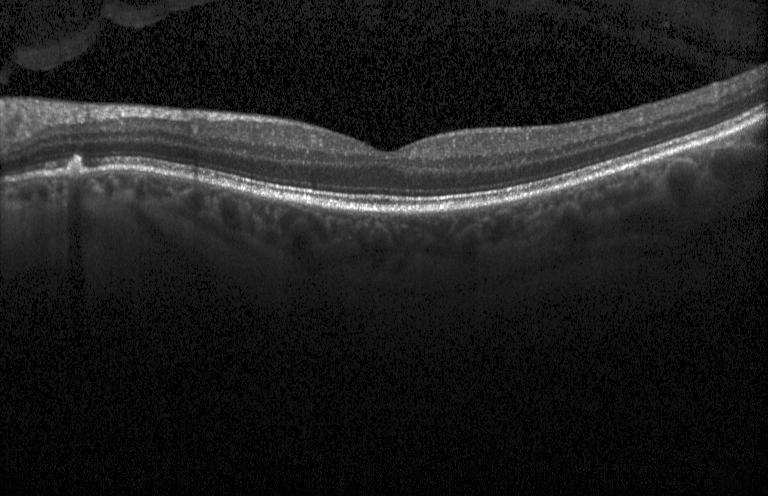
OCT scan showing no choroidal neovascularization, diabetic macular edema, or drusen.